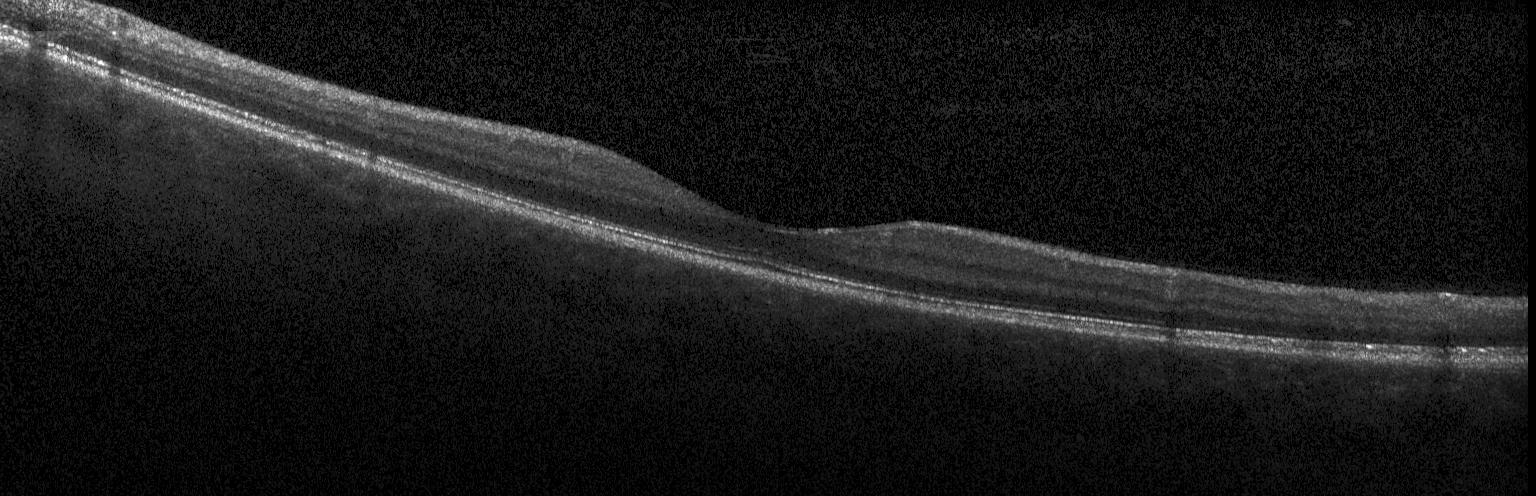

Through the macula · Heidelberg Spectralis · SD-OCT · optical coherence tomography scan
Impression: no choroidal neovascularization, no diabetic macular edema, and no drusen.